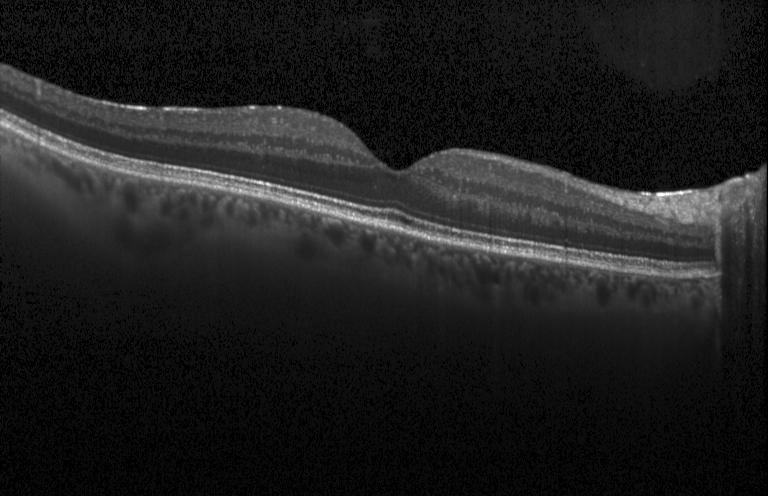 OCT B-scan showing neither choroidal neovascularization, diabetic macular edema, nor drusen.